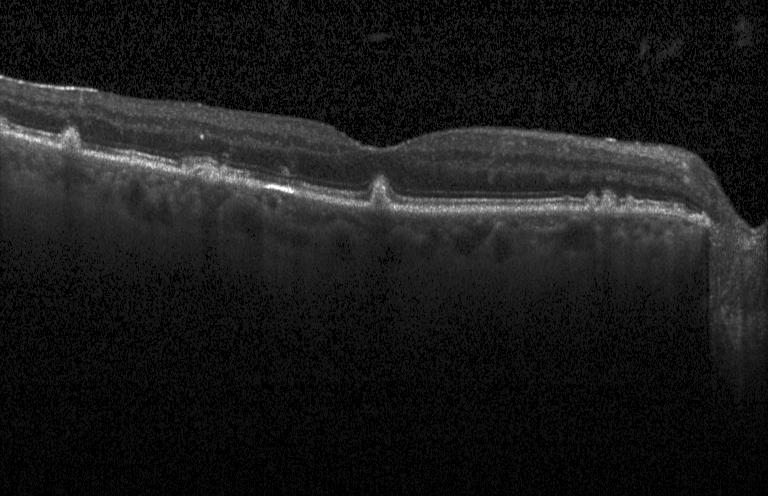
Optical coherence tomography B-scan, SD-OCT, centered on the fovea
Impression: drusen.